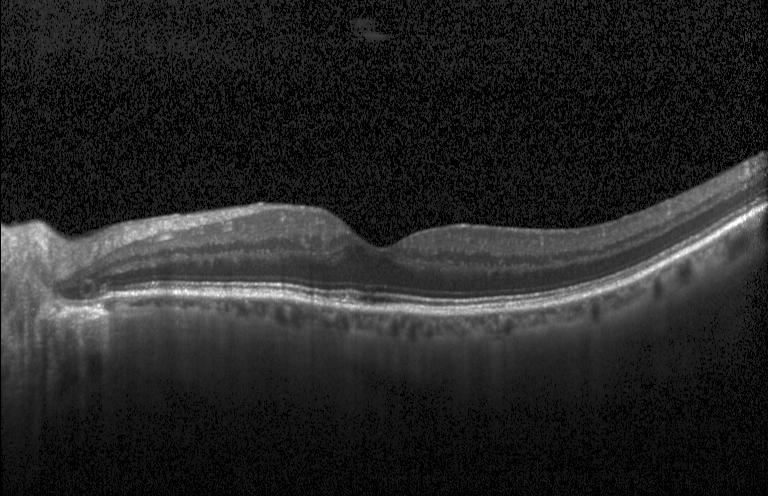
Optical coherence tomography B-scan. Fovea-centered. Spectral-domain optical coherence tomography — This B-scan demonstrates neither choroidal neovascularization, diabetic macular edema, nor drusen.